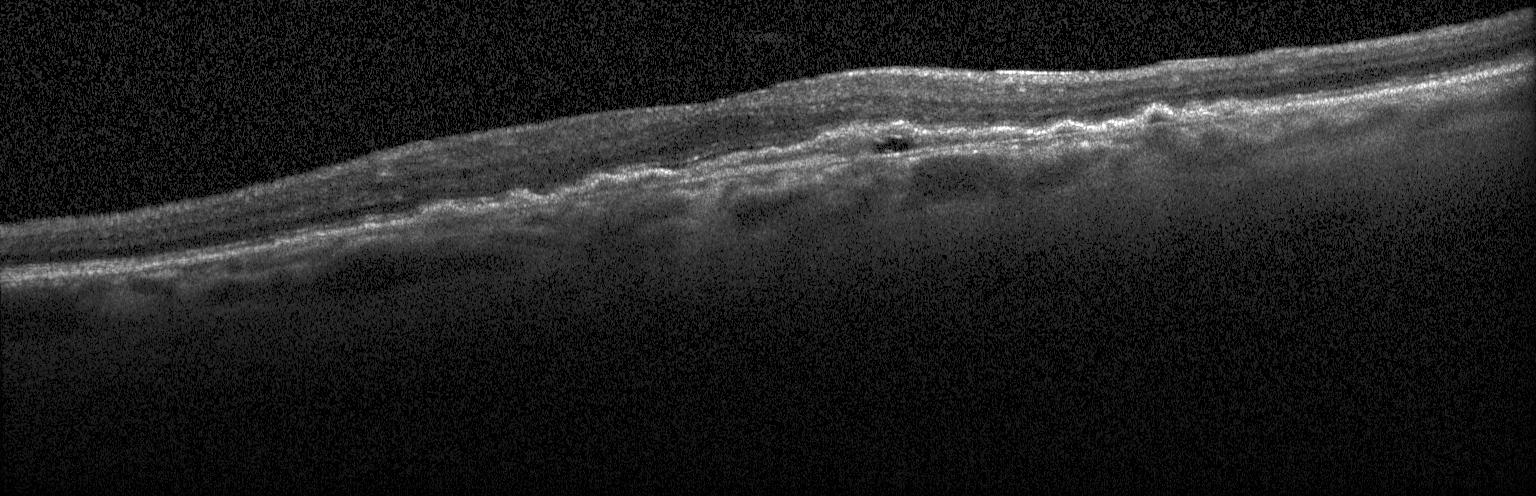 Retinal OCT cross-section; Heidelberg Spectralis; SD-OCT; fovea-centered. This B-scan demonstrates a choroidal neovascular membrane.